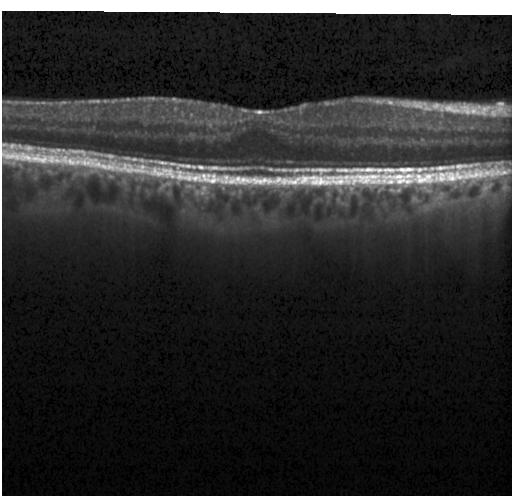
The scan shows neither choroidal neovascularization, diabetic macular edema, nor drusen.